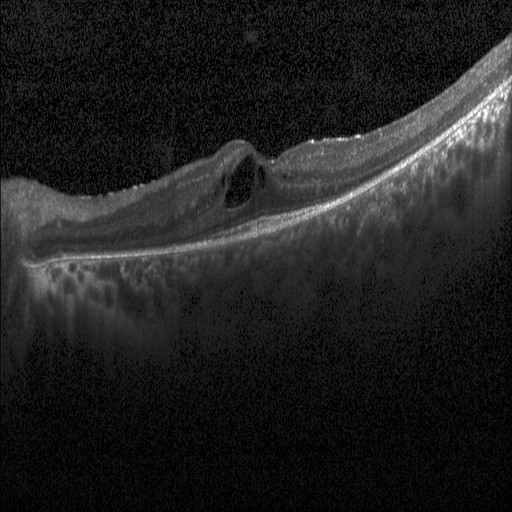 This B-scan demonstrates diabetic macular edema (DME).